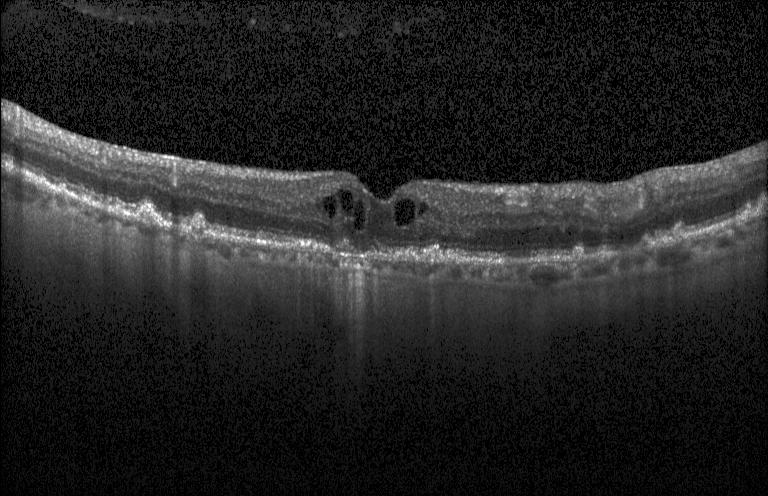

Macular scan. OCT B-scan. Spectral-domain OCT — Diagnosis: choroidal neovascularization (CNV).